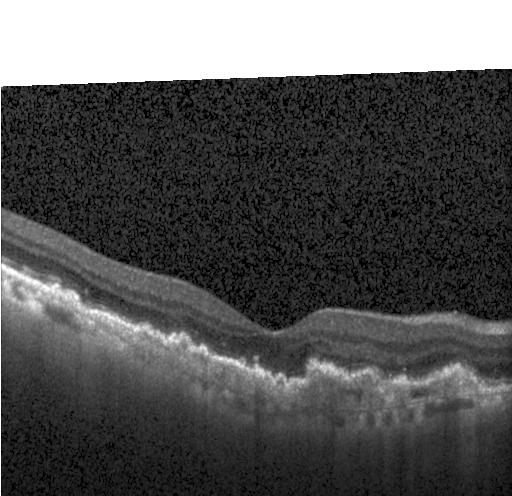

OCT scan showing choroidal neovascularization.